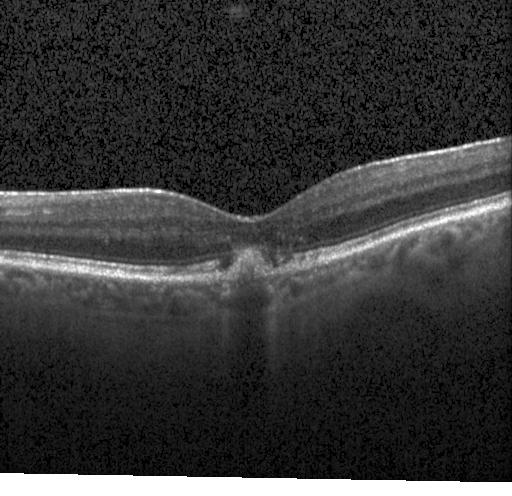 Spectral-domain OCT. Retinal OCT cross-section. Horizontal scan through the fovea. Heidelberg Spectralis OCT system.
This B-scan demonstrates CNV.